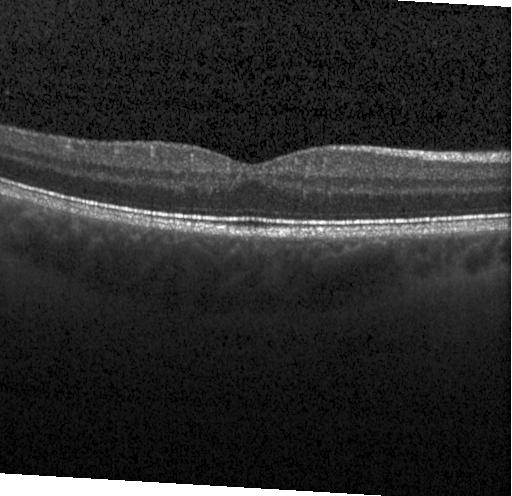

Heidelberg Spectralis OCT system, optical coherence tomography B-scan, horizontal scan through the fovea, SD-OCT.
Finding: neither choroidal neovascularization, diabetic macular edema, nor drusen.